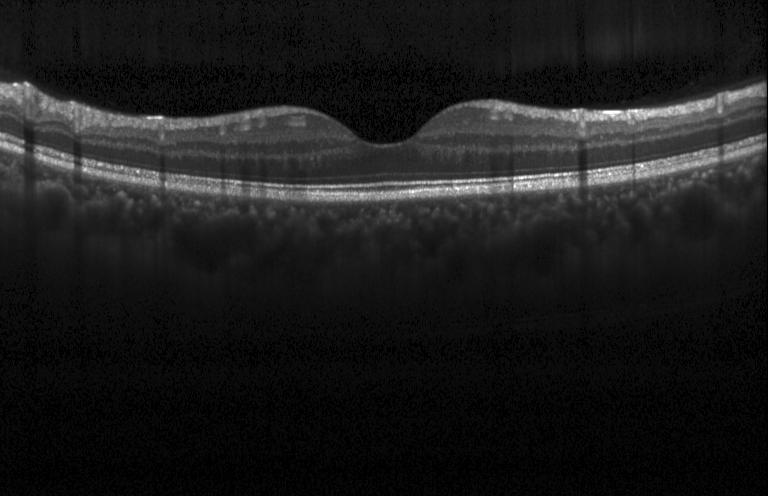
OCT B-scan showing no CNV, no DME, and no drusen.